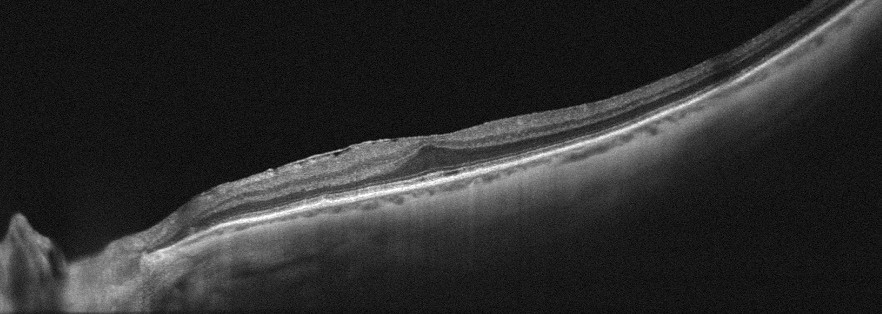 Optovue Avanti RTVue XR · optical coherence tomography B-scan. Assessment: epiretinal membrane (ERM).